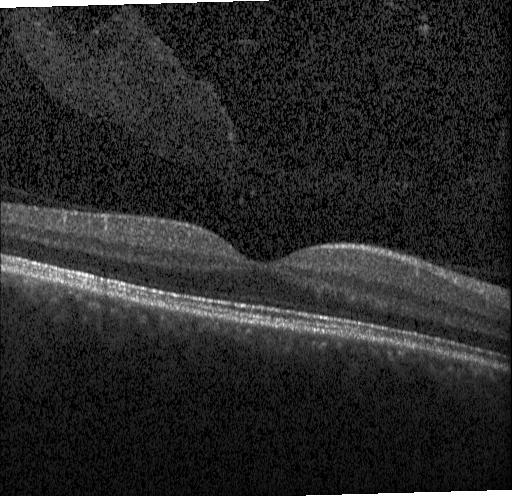

Dx: no evidence of choroidal neovascularization, diabetic macular edema, or drusen.